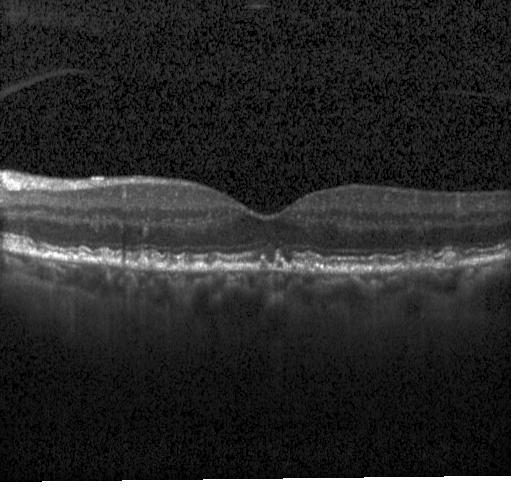 OCT B-scan; Heidelberg Spectralis; macular scan; SD-OCT.
This B-scan demonstrates sub-RPE drusenoid deposits.